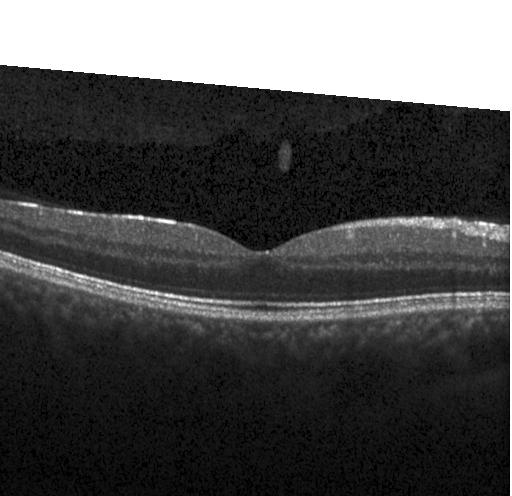
Retinal OCT cross-section. Heidelberg Spectralis. Macular scan. The scan shows no CNV, no DME, and no drusen.